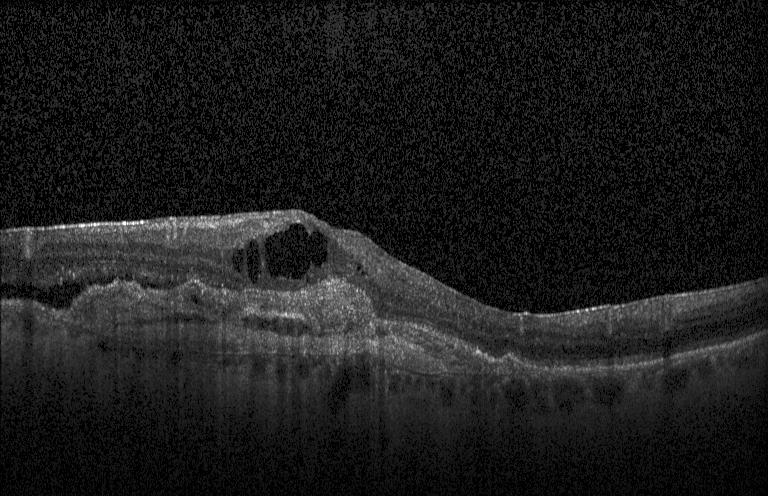
Diagnosis: a choroidal neovascular membrane.